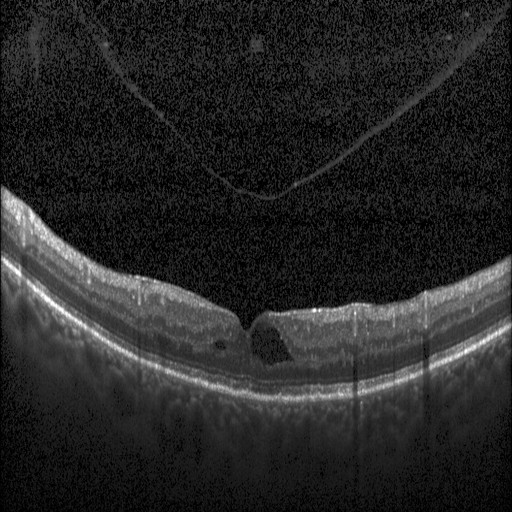
Macular OCT: diabetic macular edema.